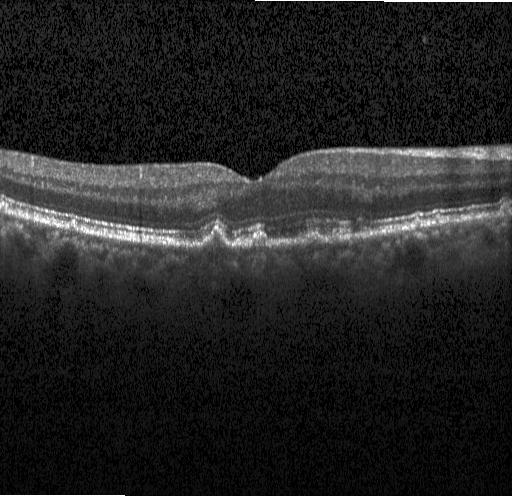

OCT finding: drusen.